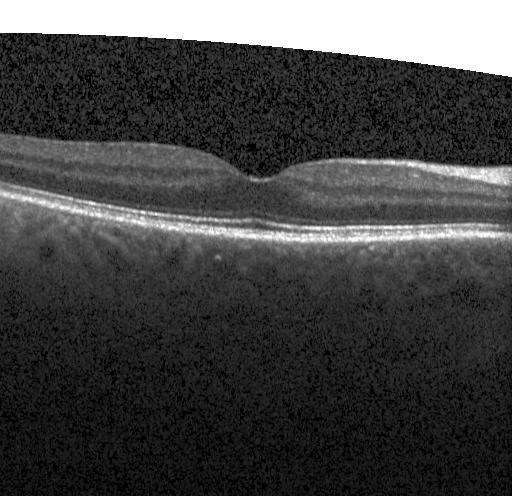

Acquired on a Heidelberg Spectralis · optical coherence tomography B-scan. This B-scan demonstrates no choroidal neovascularization, no diabetic macular edema, and no drusen.